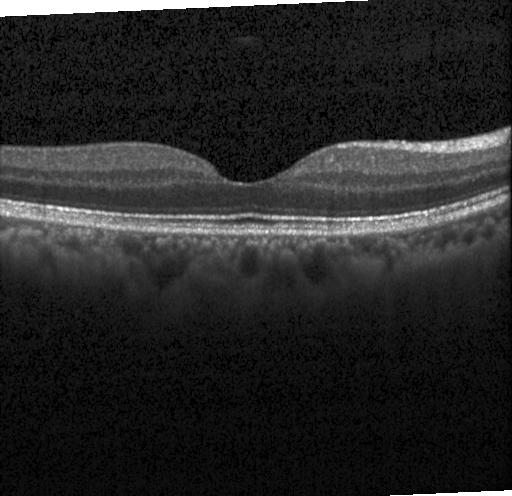

Retinal OCT B-scan
Assessment: no choroidal neovascularization, no diabetic macular edema, and no drusen.